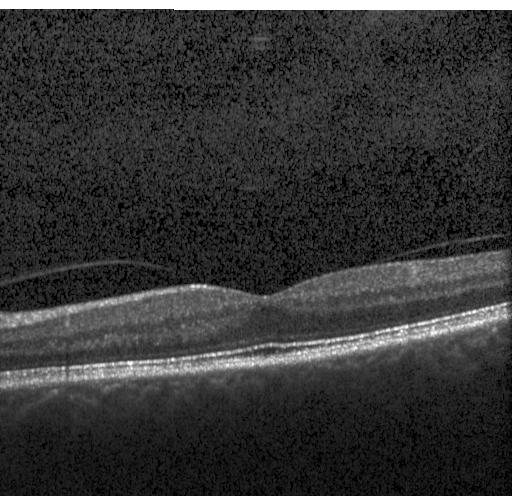
Diagnosis: no CNV, no DME, and no drusen.